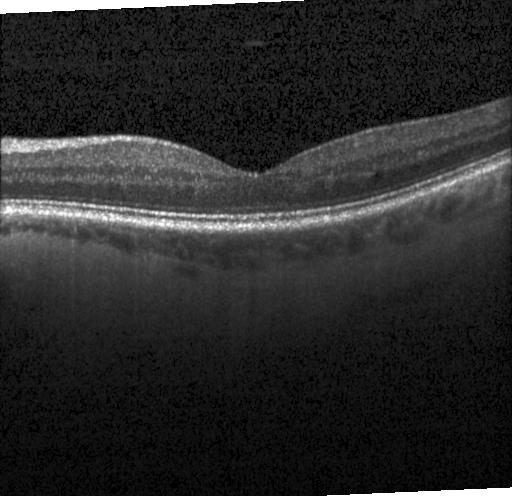 Acquired on a Heidelberg Spectralis; OCT B-scan.
No choroidal neovascularization, diabetic macular edema, or drusen.